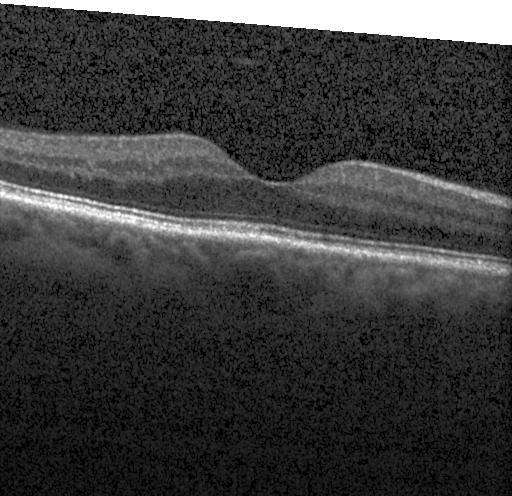
OCT line scan.
Dx: no CNV, no DME, and no drusen.